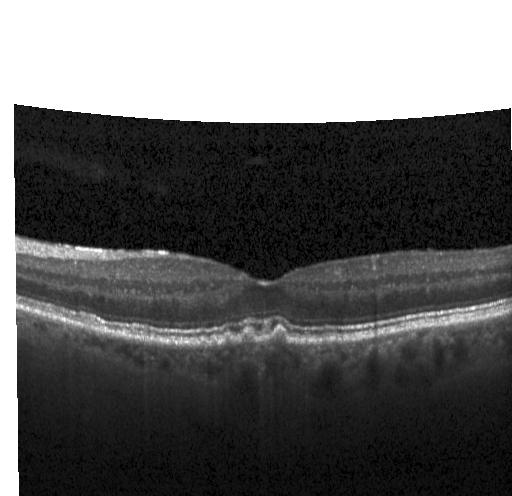
OCT B-scan, Heidelberg Spectralis, fovea-centered
Macular OCT: drusen.